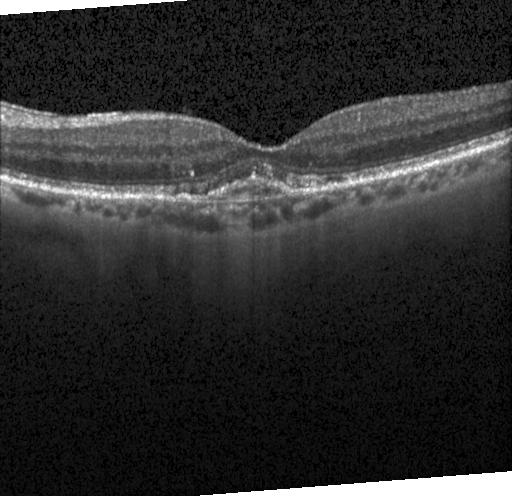
Optical coherence tomography scan; centered on the fovea.
The scan shows a choroidal neovascular membrane.